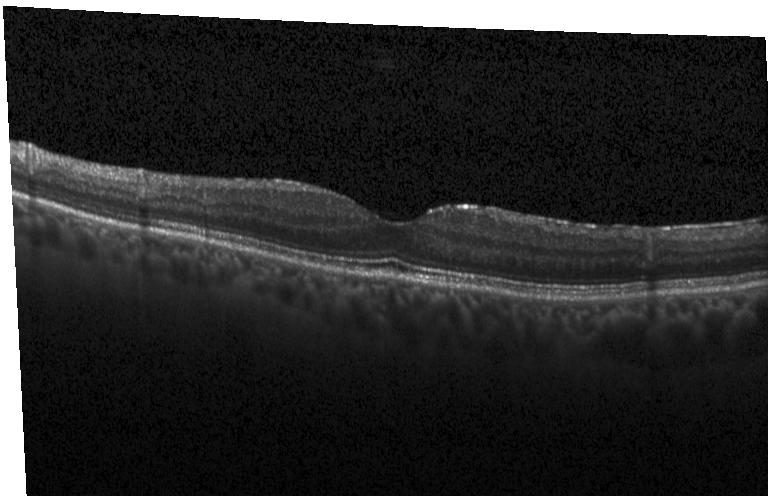 Instrument: Heidelberg Spectralis; OCT line scan; through the macula
Diagnosis: no CNV, no DME, and no drusen.